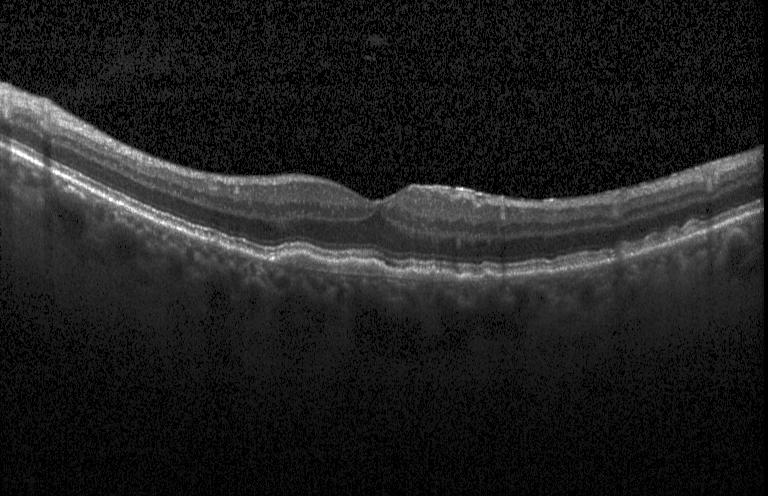

Heidelberg Spectralis OCT system. Optical coherence tomography B-scan. Finding: CNV.